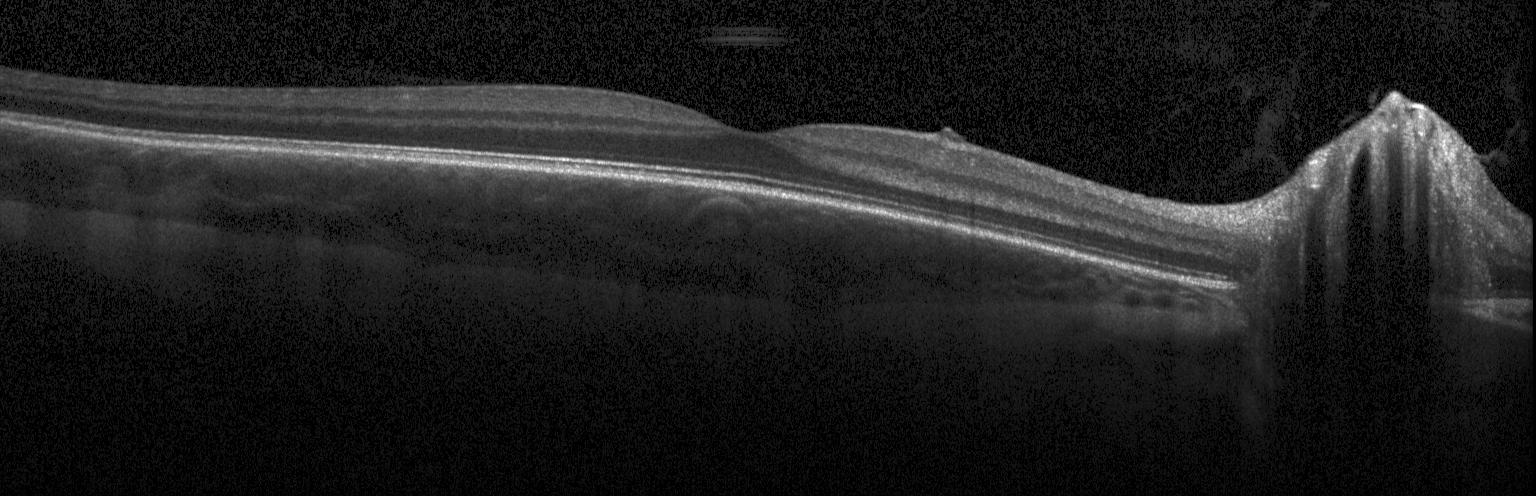
Retinal OCT B-scan. The scan shows no CNV, no DME, and no drusen.